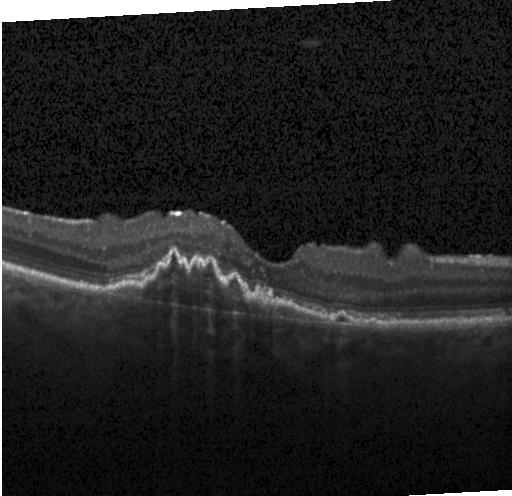 Optical coherence tomography B-scan
This B-scan demonstrates a choroidal neovascular membrane.